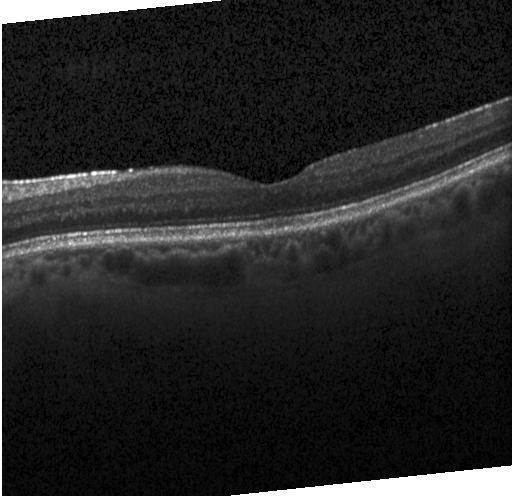

Fovea-centered; spectral-domain optical coherence tomography; retinal OCT B-scan; Heidelberg Spectralis.
The scan shows no evidence of choroidal neovascularization, diabetic macular edema, or drusen.